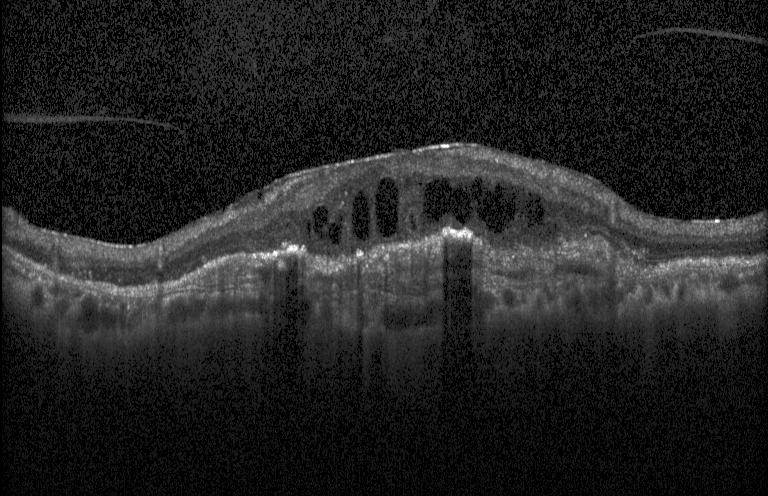

Retinal OCT B-scan; macular scan; spectral-domain OCT; instrument: Heidelberg Spectralis — OCT finding: CNV.